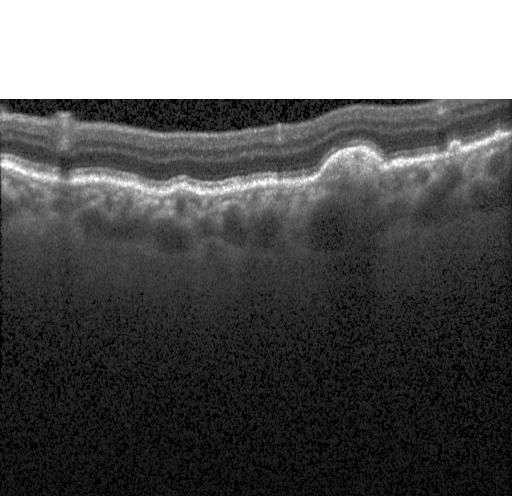 Optical coherence tomography scan.
OCT finding: drusen.